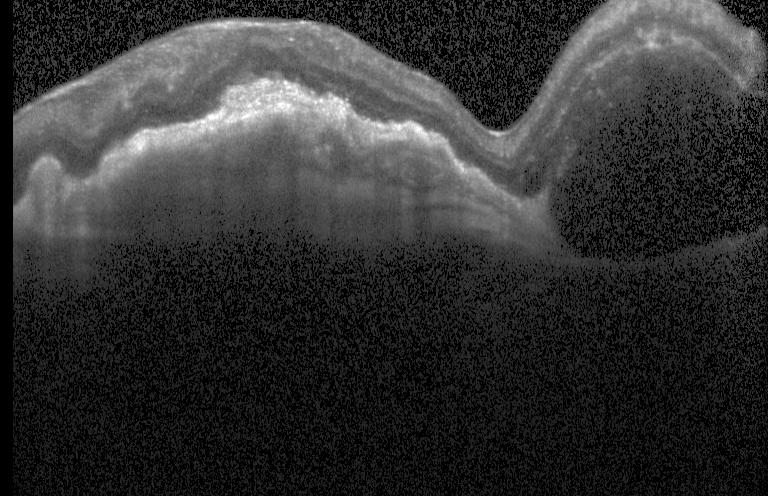 Assessment: CNV.